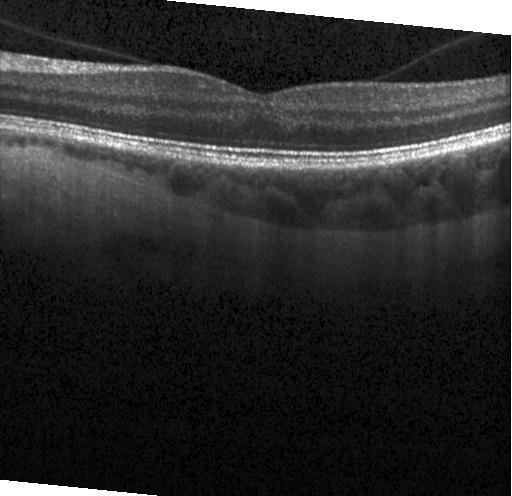
Optical coherence tomography B-scan. Impression: no evidence of CNV, DME, or drusen.